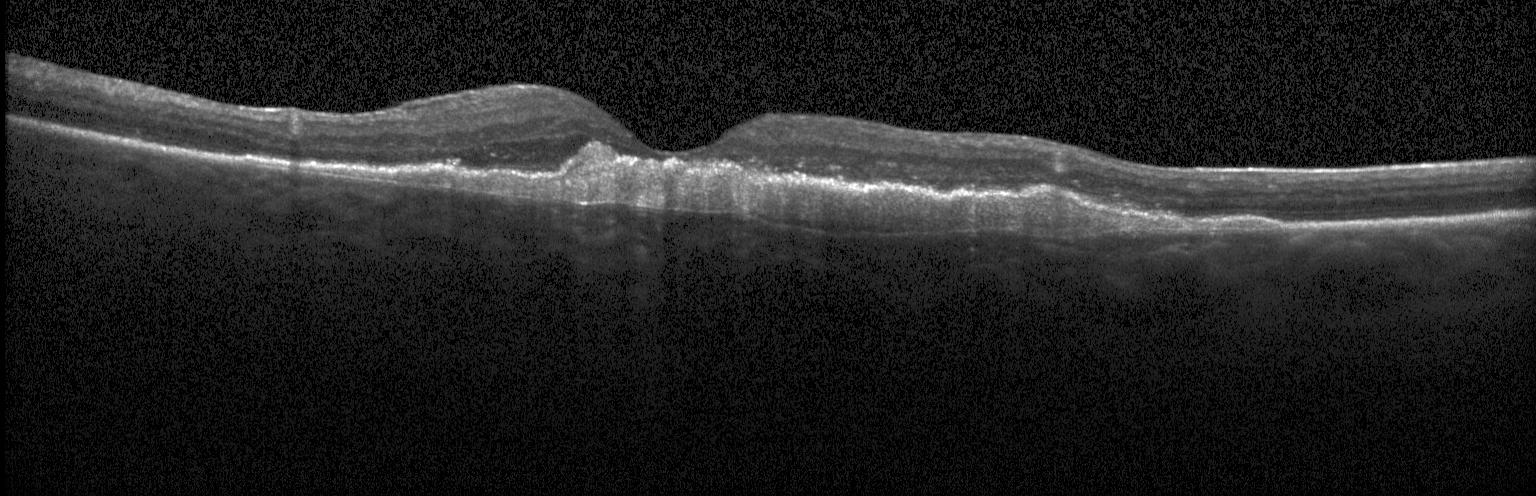

Assessment: CNV.